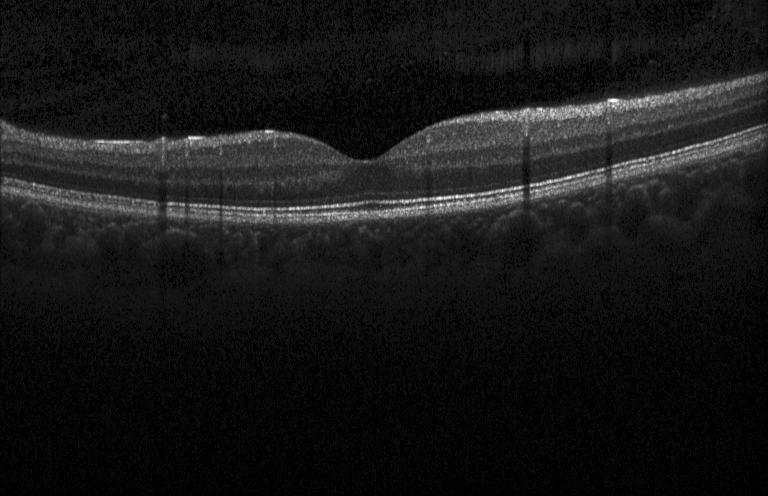
Retinal OCT cross-section. SD-OCT. Macular scan
OCT finding: no choroidal neovascularization, no diabetic macular edema, and no drusen.